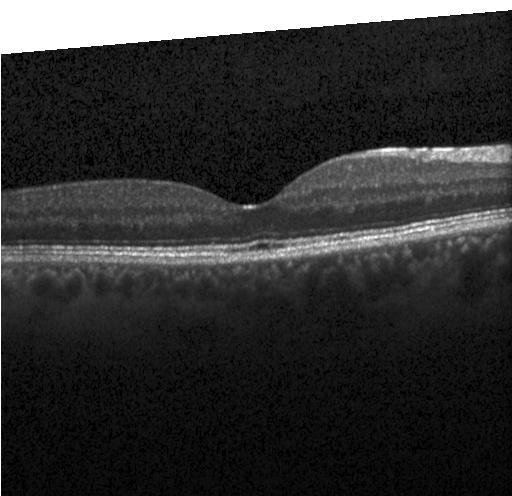 Dx: no CNV, DME, or drusen.